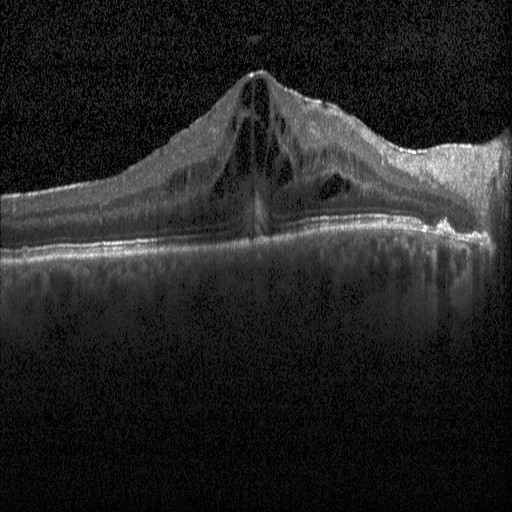

Retinal OCT B-scan. Heidelberg Spectralis OCT system. Macular scan. Spectral-domain optical coherence tomography. Assessment: DME.